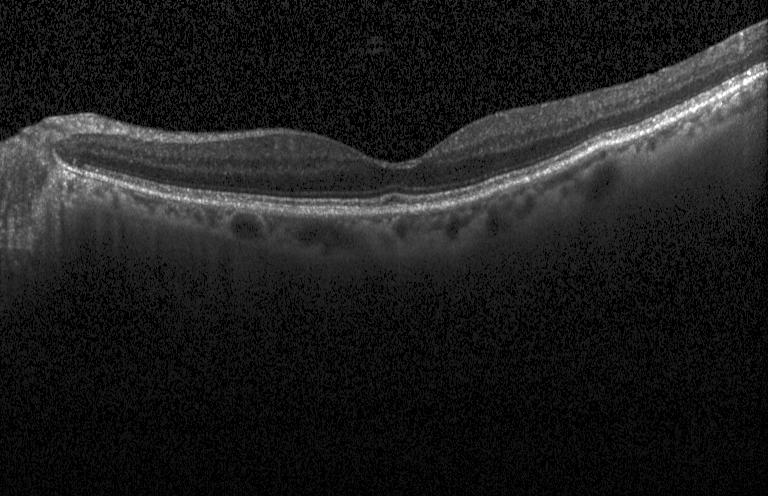 Impression: no choroidal neovascularization, diabetic macular edema, or drusen.